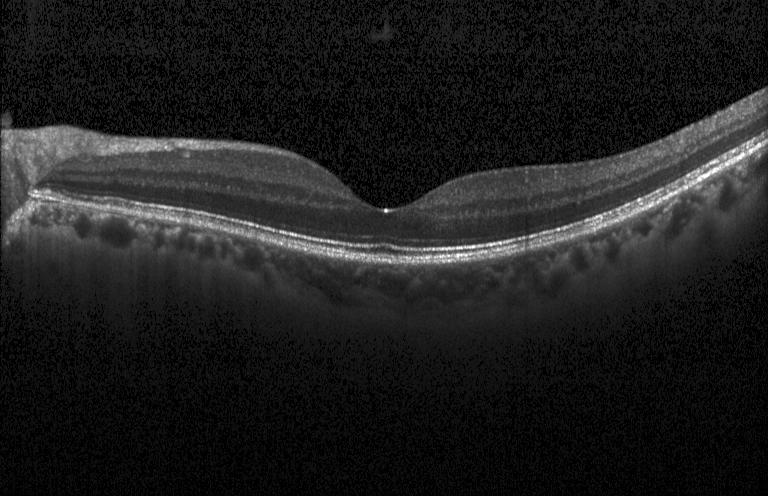 Optical coherence tomography scan. Spectral-domain optical coherence tomography.
Dx: neither CNV, DME, nor drusen.